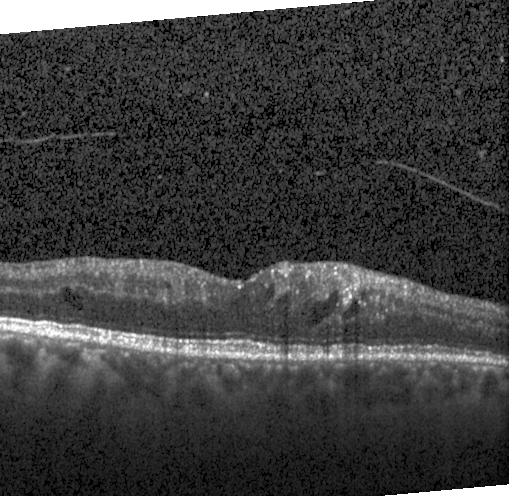

Spectral-domain OCT; retinal OCT B-scan — Diagnosis: diabetic macular edema.